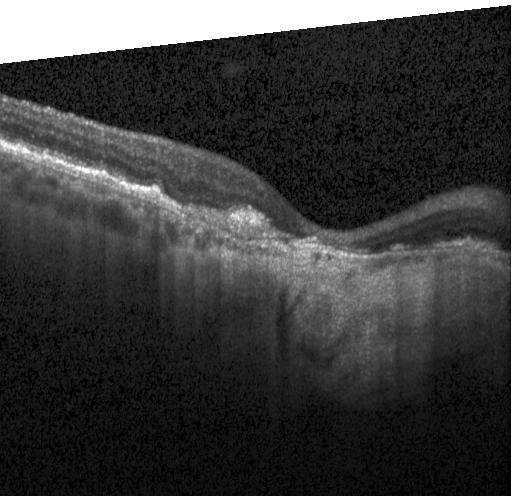 Centered on the fovea. Optical coherence tomography B-scan. Acquired on a Heidelberg Spectralis
Assessment: a choroidal neovascular membrane.